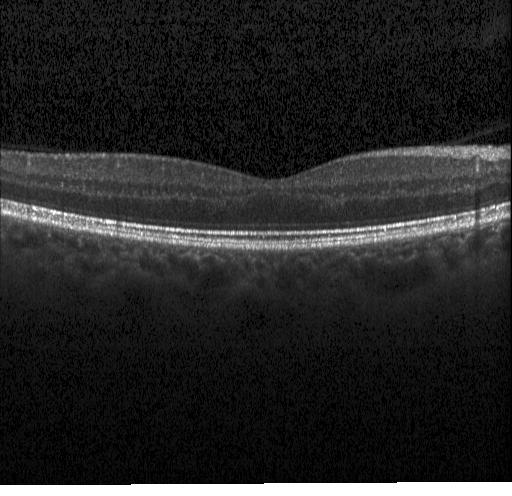
Centered on the fovea; OCT line scan. This B-scan demonstrates neither CNV, DME, nor drusen.